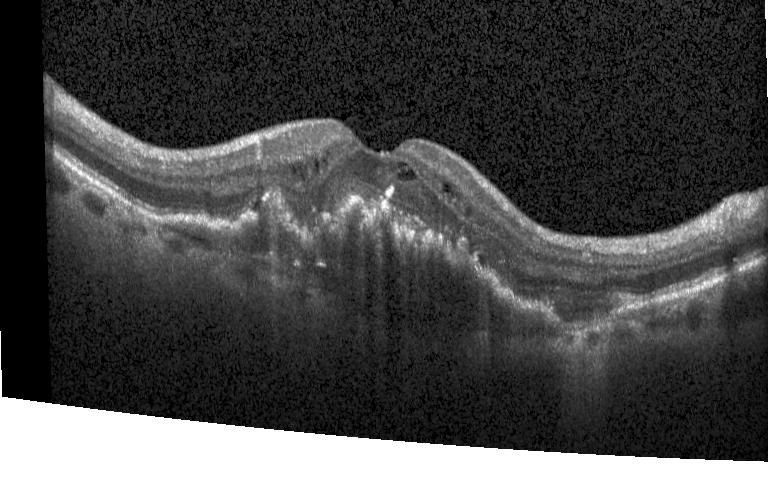

Diagnosis: a choroidal neovascular membrane.